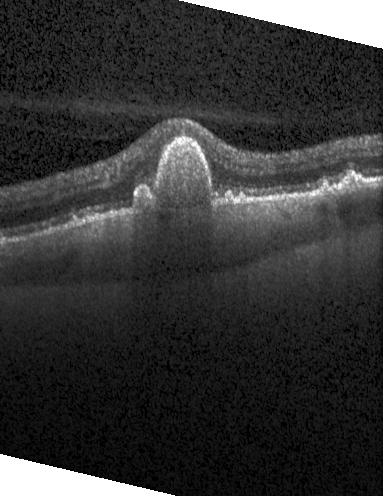 Finding: CNV.